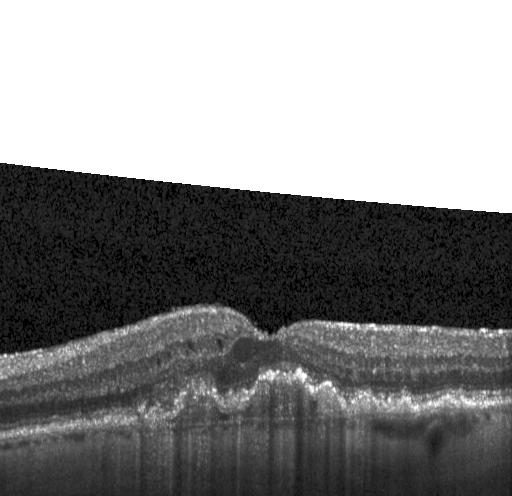 A choroidal neovascular membrane.